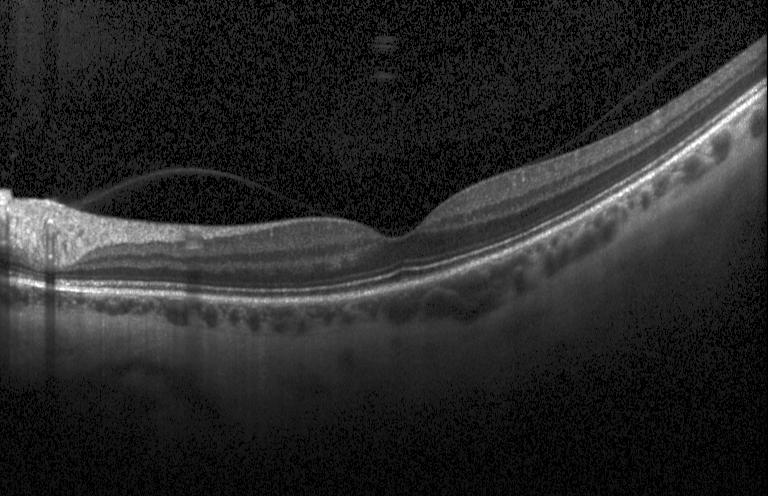

Retinal OCT cross-section — Macular OCT: neither choroidal neovascularization, diabetic macular edema, nor drusen.